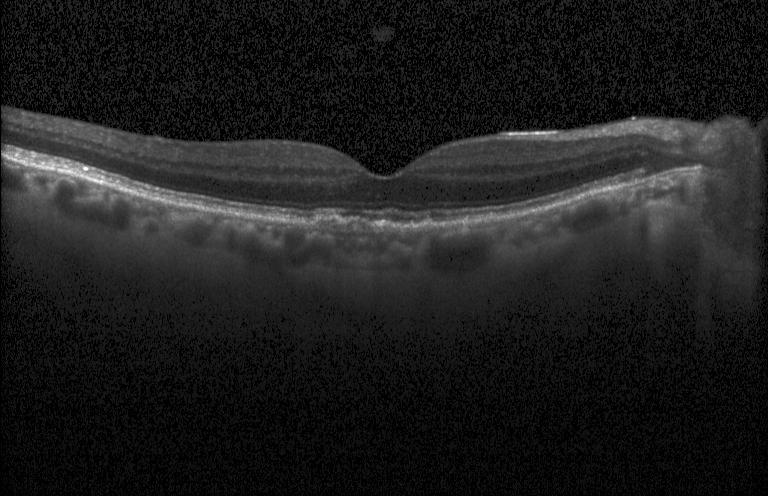

OCT B-scan showing sub-RPE drusenoid deposits.